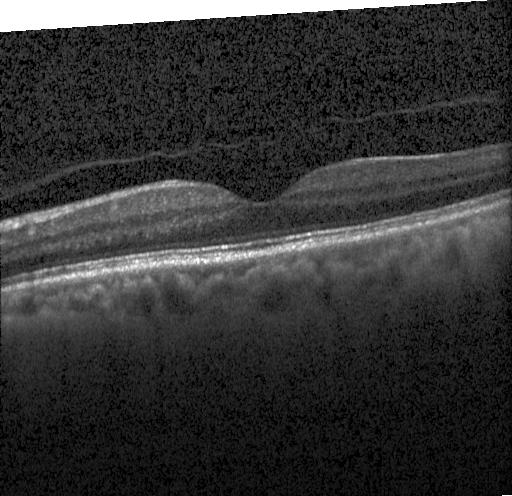
Optical coherence tomography scan, fovea-centered, Heidelberg Spectralis OCT system
Assessment: no choroidal neovascularization, diabetic macular edema, or drusen.